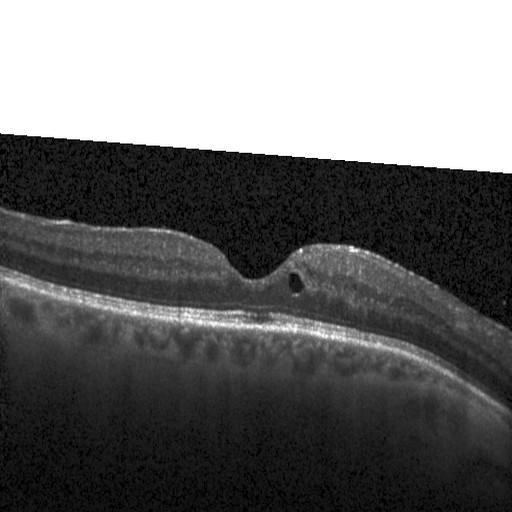

Impression: diabetic macular edema.